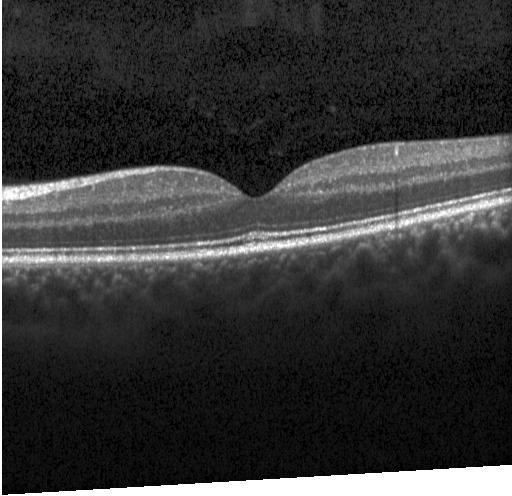
OCT finding: no evidence of choroidal neovascularization, diabetic macular edema, or drusen.